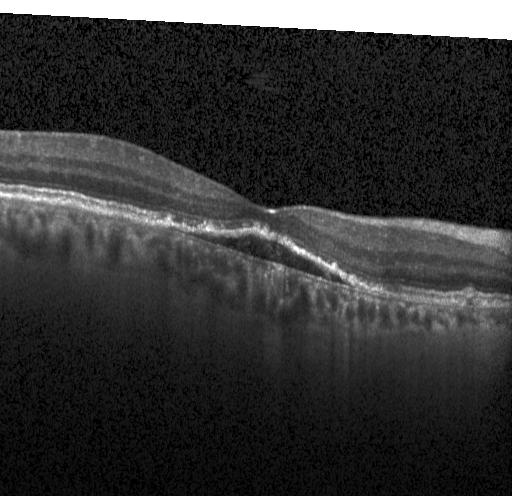

Optical coherence tomography B-scan. The scan shows a choroidal neovascular membrane.